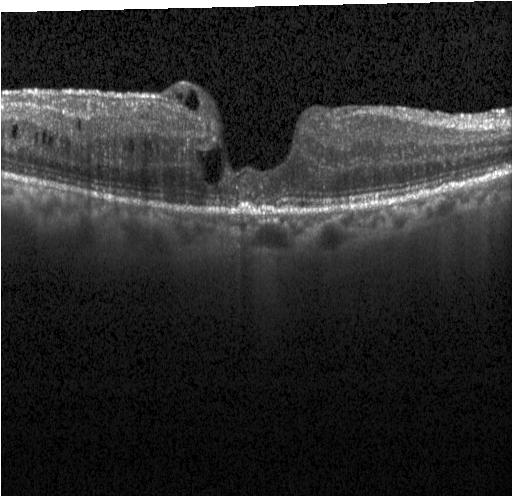

Impression: diabetic macular edema (DME).